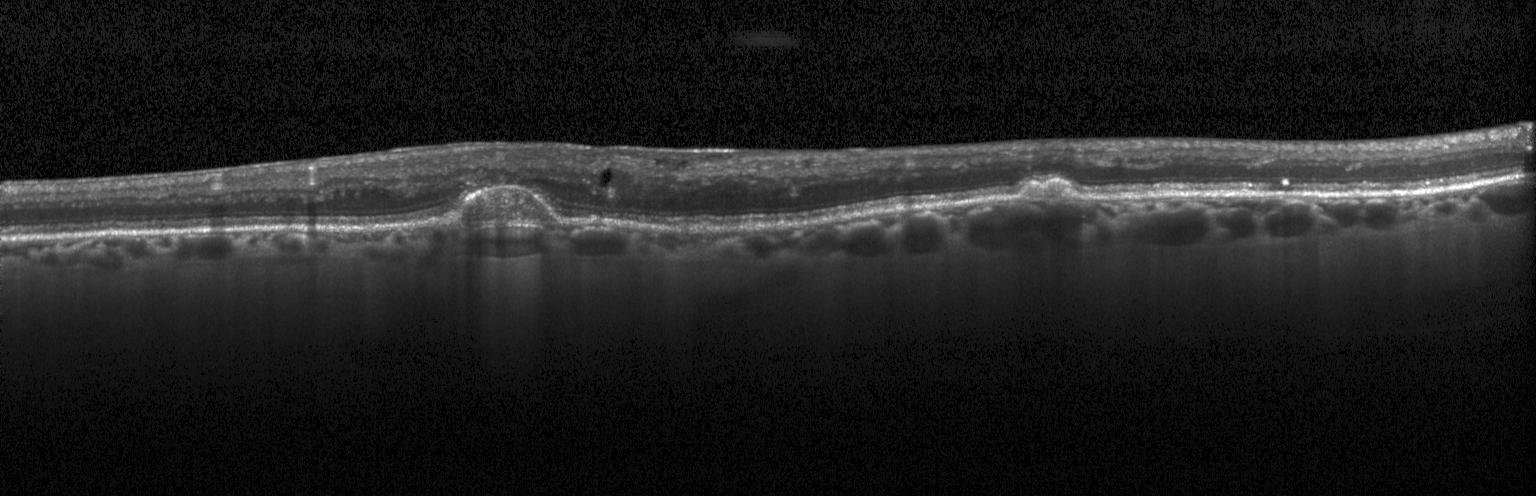
Spectral-domain OCT, Heidelberg Spectralis, macular scan, optical coherence tomography scan
Macular OCT: choroidal neovascularization (CNV).